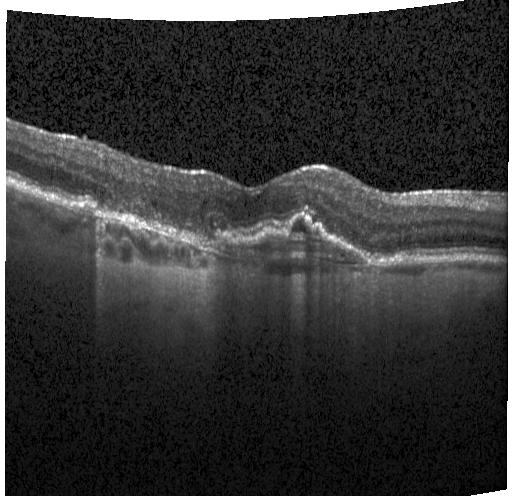
OCT finding: a choroidal neovascular membrane.